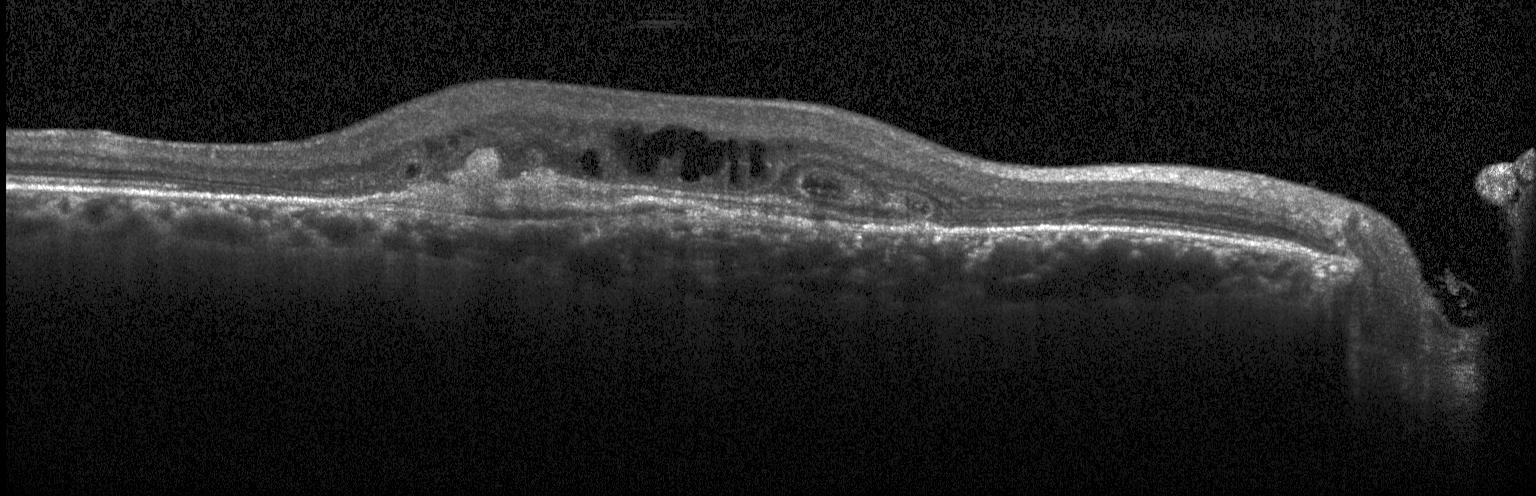
Diagnosis: choroidal neovascularization.